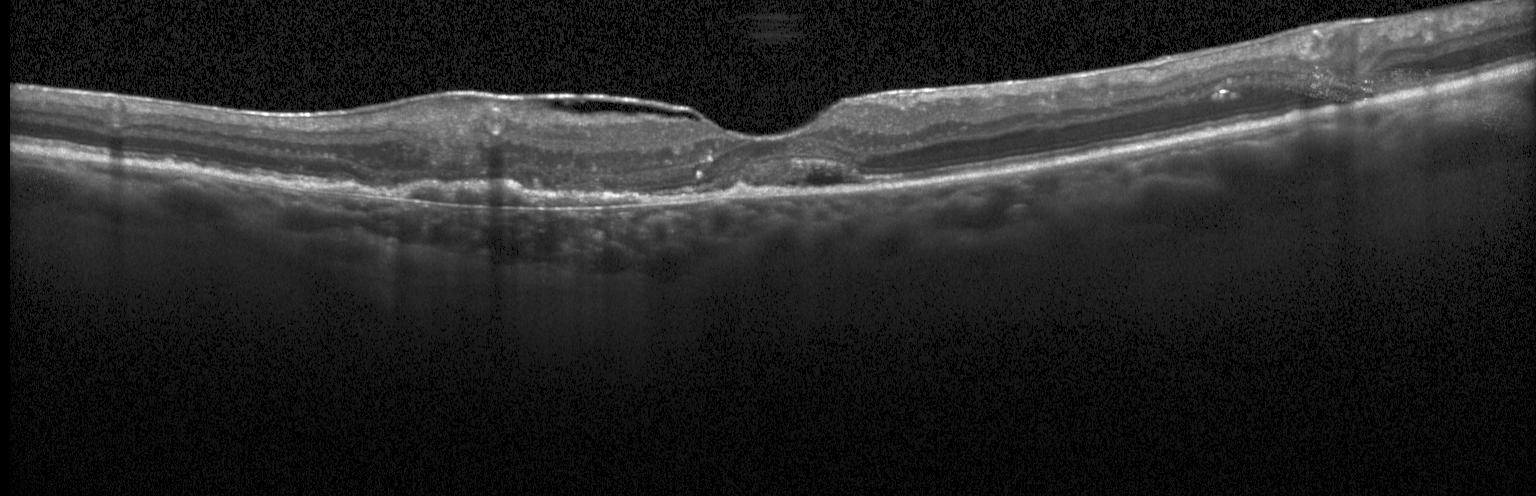
Retinal OCT cross-section.
Impression: a choroidal neovascular membrane.